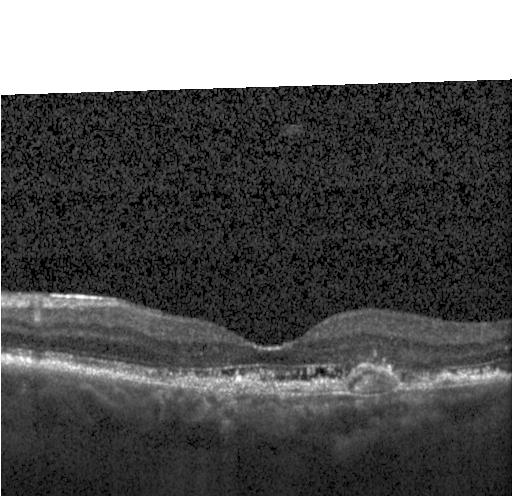
Instrument: Heidelberg Spectralis; SD-OCT; centered on the fovea; optical coherence tomography scan
The scan shows choroidal neovascularization (CNV).